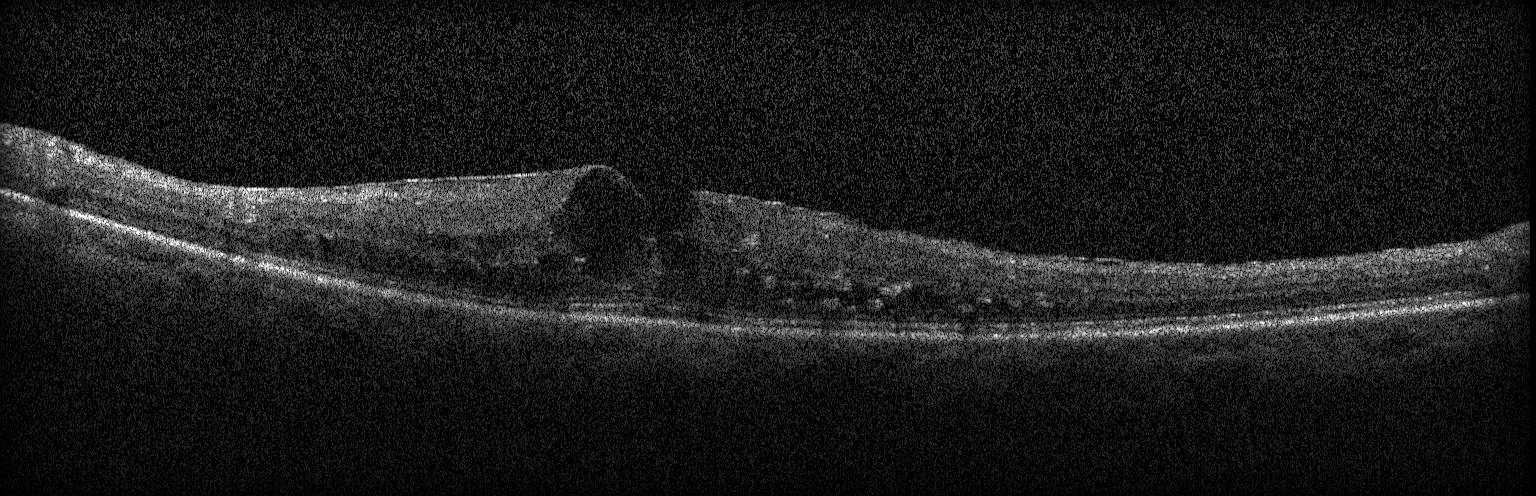
Retinal OCT B-scan.
Impression: DME.